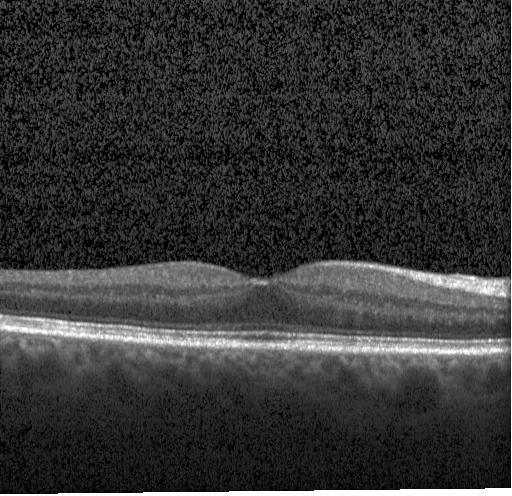 OCT B-scan showing no choroidal neovascularization, diabetic macular edema, or drusen.